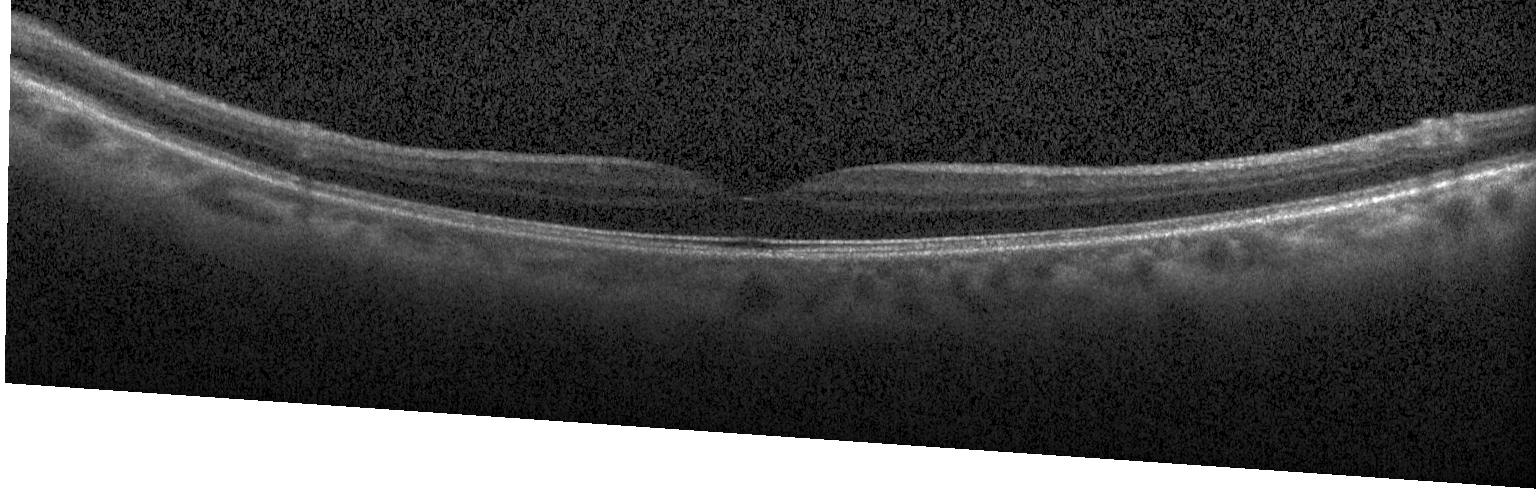 Macular OCT demonstrating neither CNV, DME, nor drusen.